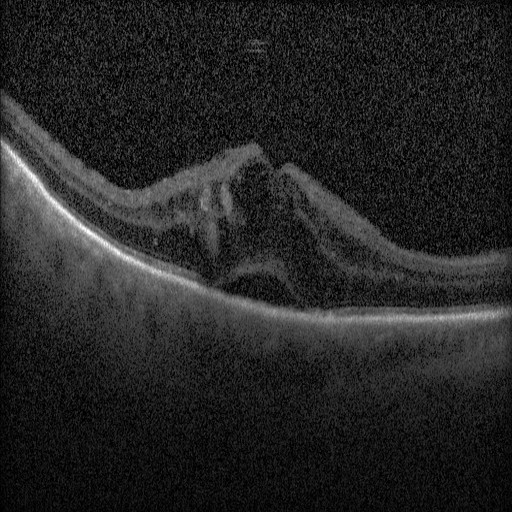

SD-OCT · OCT B-scan · through the macula — Finding: diabetic macular edema (DME).